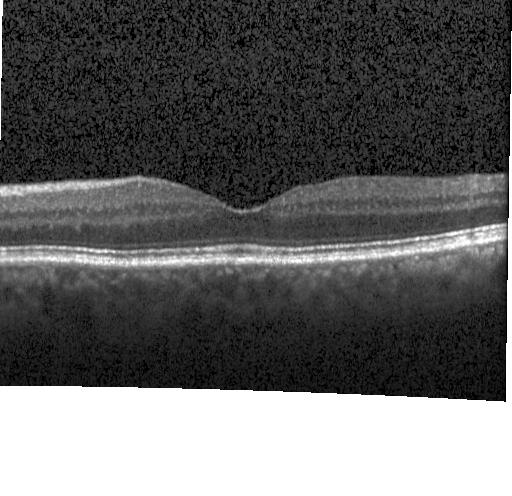
Optical coherence tomography B-scan
The scan shows no choroidal neovascularization, no diabetic macular edema, and no drusen.